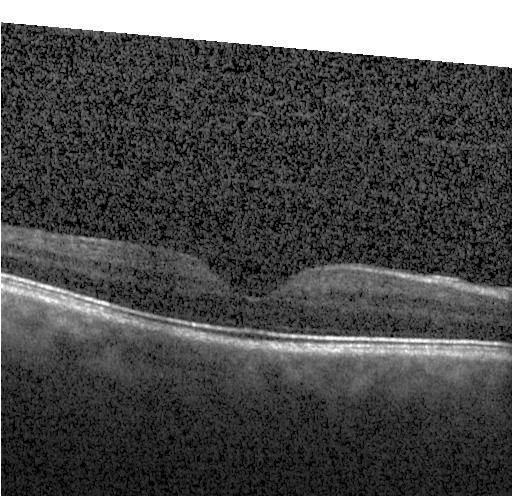 Spectral-domain OCT B-scan: no choroidal neovascularization, no diabetic macular edema, and no drusen.